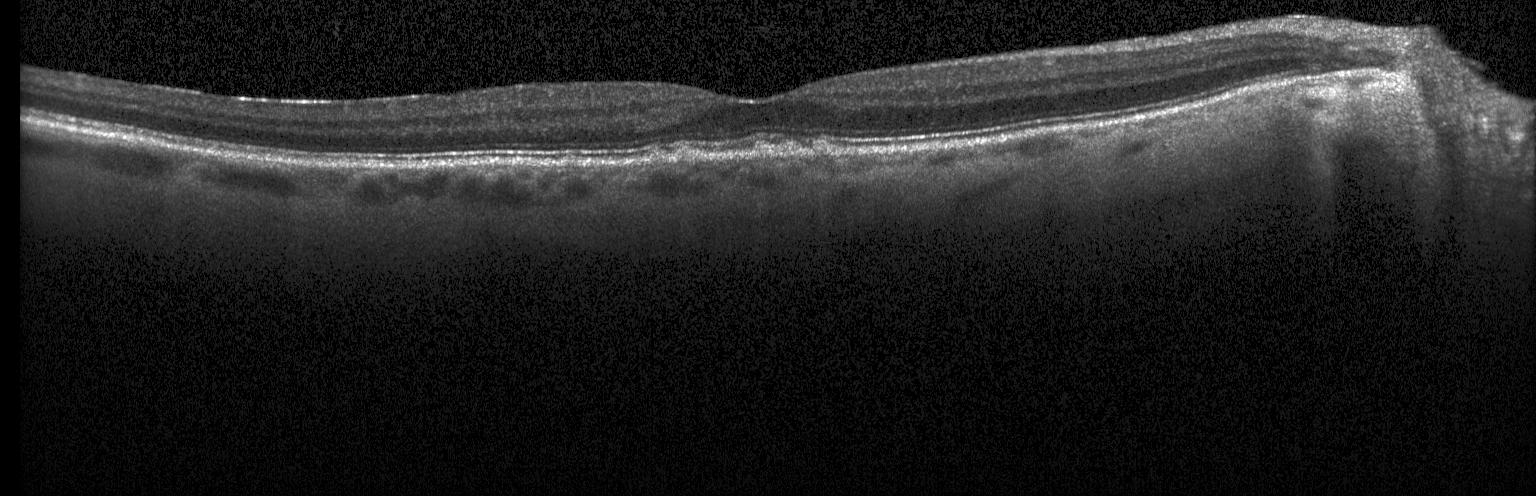 OCT finding: multiple drusen.